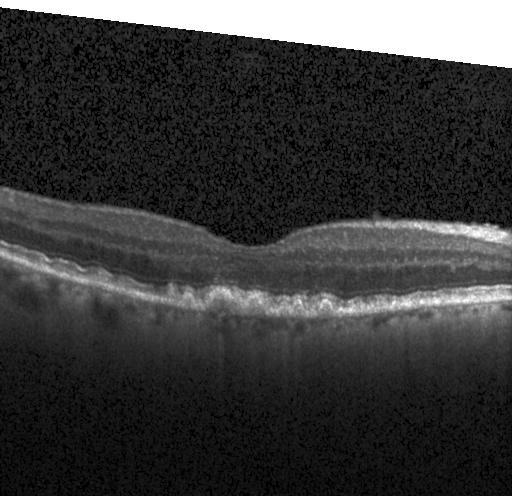
Retinal OCT B-scan
Finding: multiple drusen.